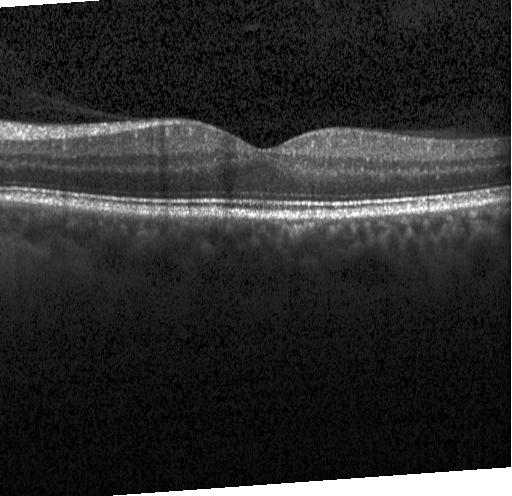 Optical coherence tomography scan — The scan shows no choroidal neovascularization, no diabetic macular edema, and no drusen.